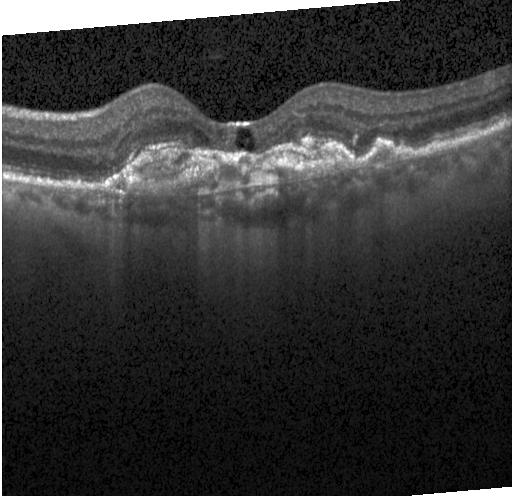
Retinal OCT cross-section
CNV.